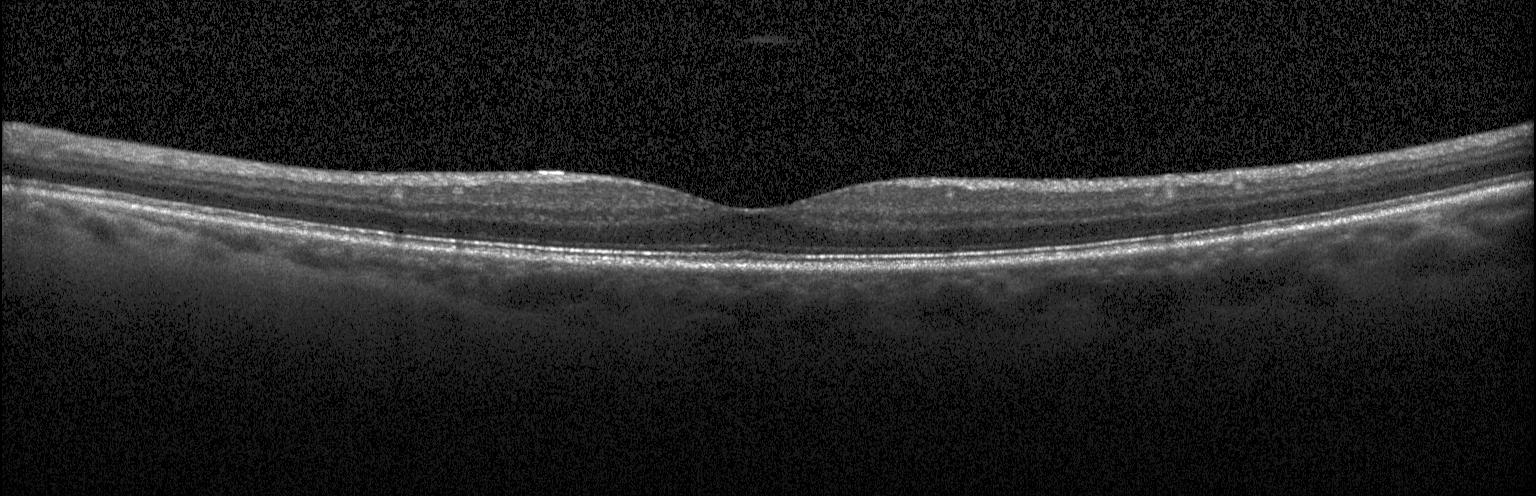 Assessment: no evidence of choroidal neovascularization, diabetic macular edema, or drusen.